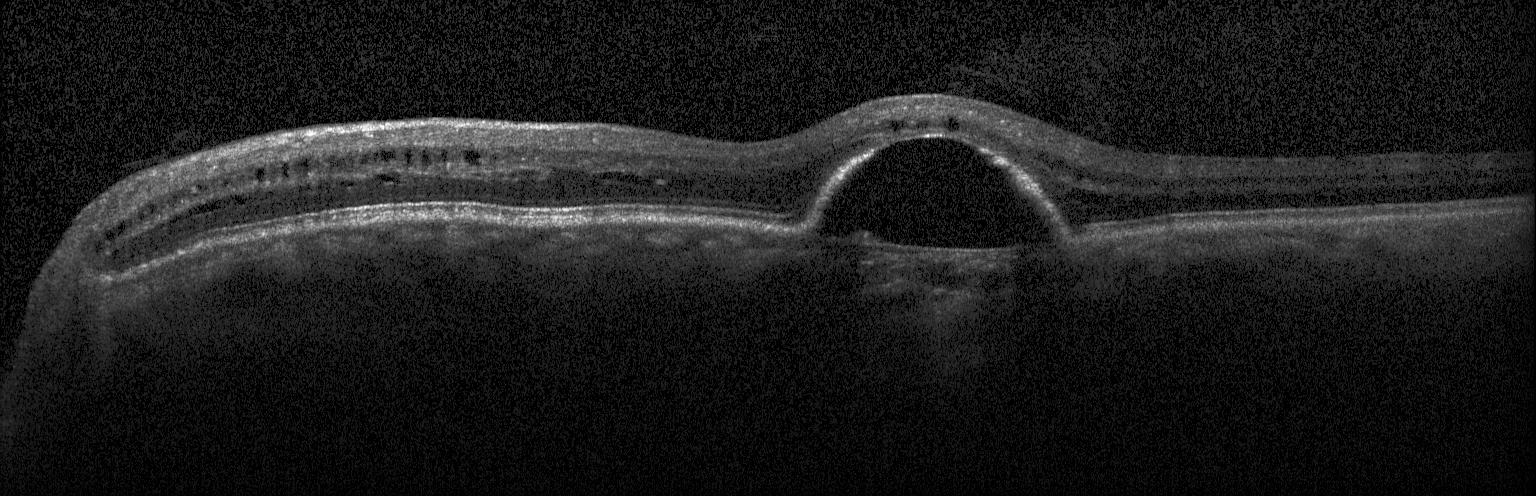
Instrument: Heidelberg Spectralis. Optical coherence tomography B-scan
Impression: a choroidal neovascular membrane.